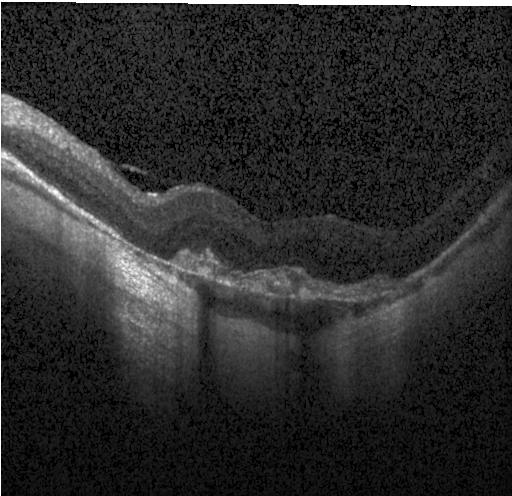 Centered on the fovea, optical coherence tomography scan — Impression: CNV.